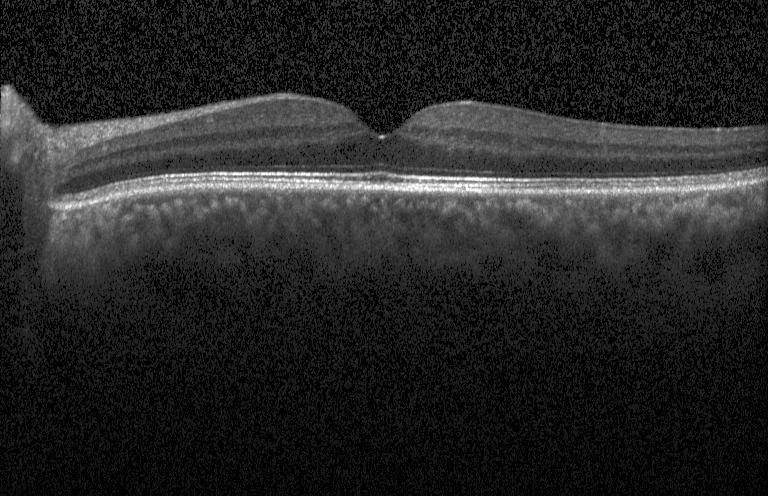

Fovea-centered; retinal OCT cross-section; Heidelberg Spectralis; spectral-domain optical coherence tomography. The scan shows no choroidal neovascularization, diabetic macular edema, or drusen.